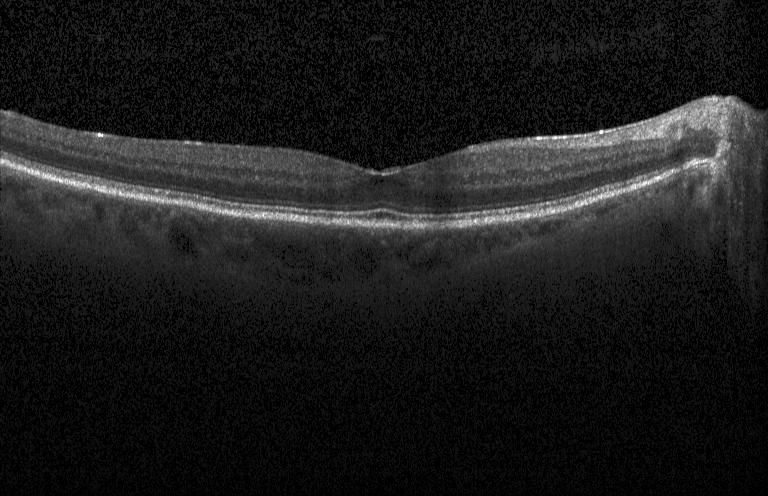
Optical coherence tomography B-scan; acquired on a Heidelberg Spectralis.
This B-scan demonstrates no CNV, no DME, and no drusen.